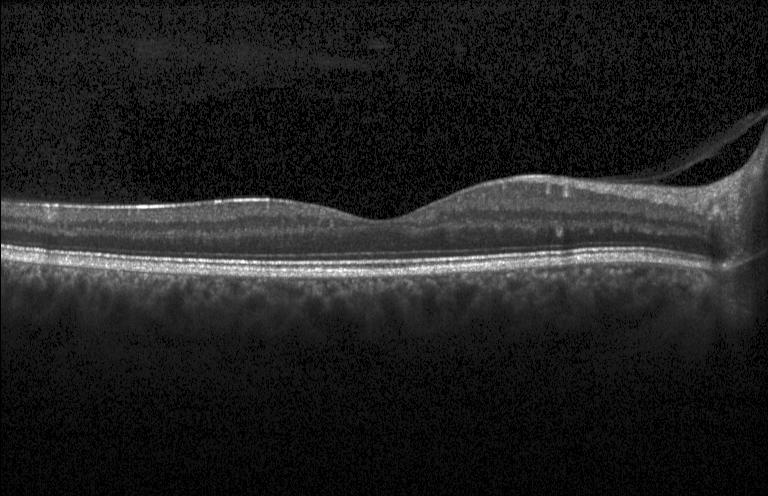
Spectral-domain OCT B-scan: no evidence of choroidal neovascularization, diabetic macular edema, or drusen.